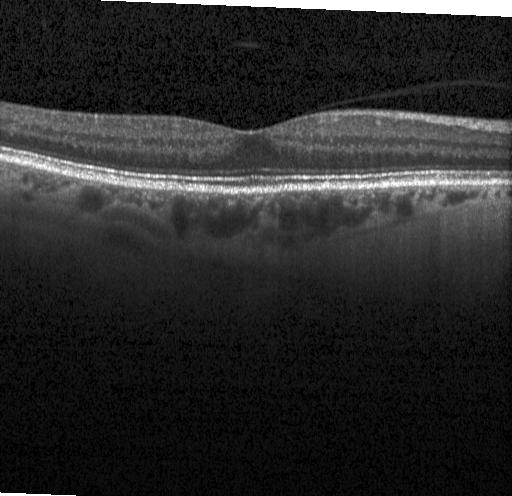 OCT line scan · through the macula. Macular OCT: no choroidal neovascularization, diabetic macular edema, or drusen.